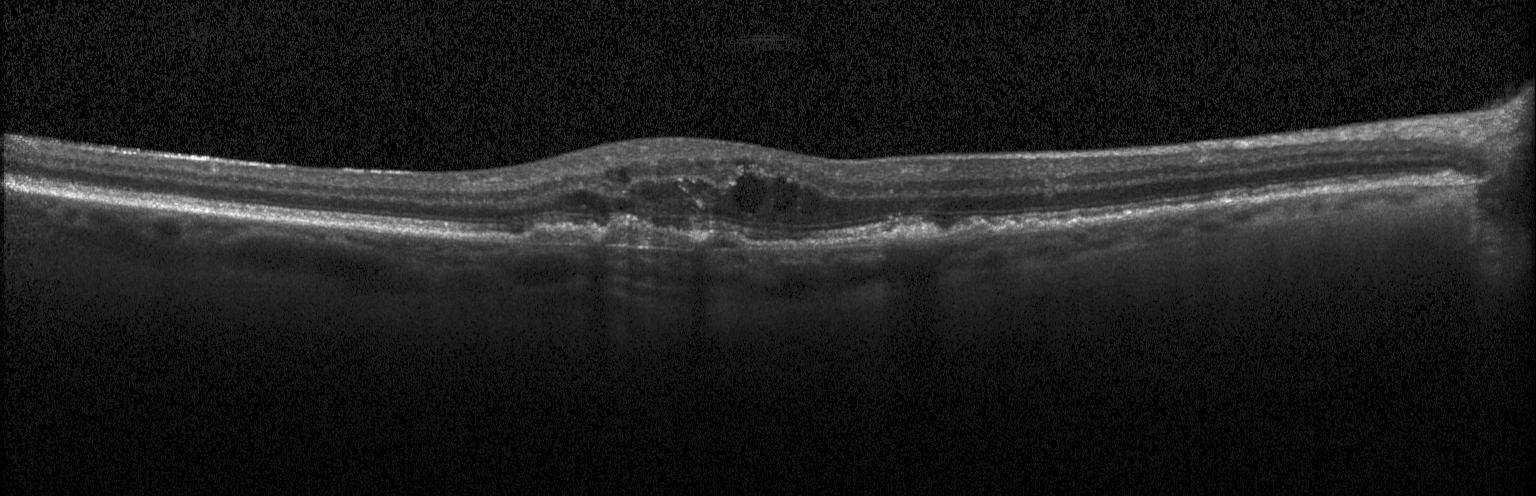
Impression: a choroidal neovascular membrane.